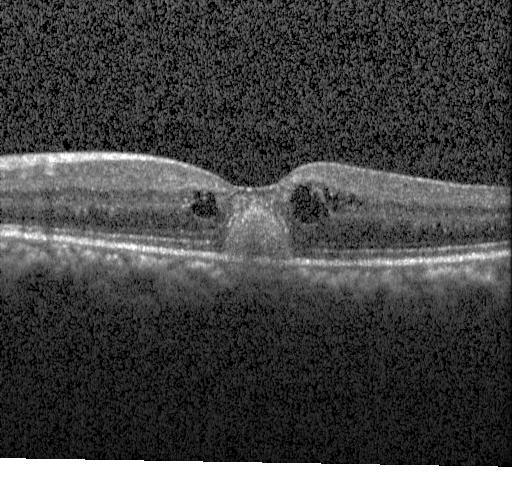
Optical coherence tomography B-scan. Macular OCT: a choroidal neovascular membrane.